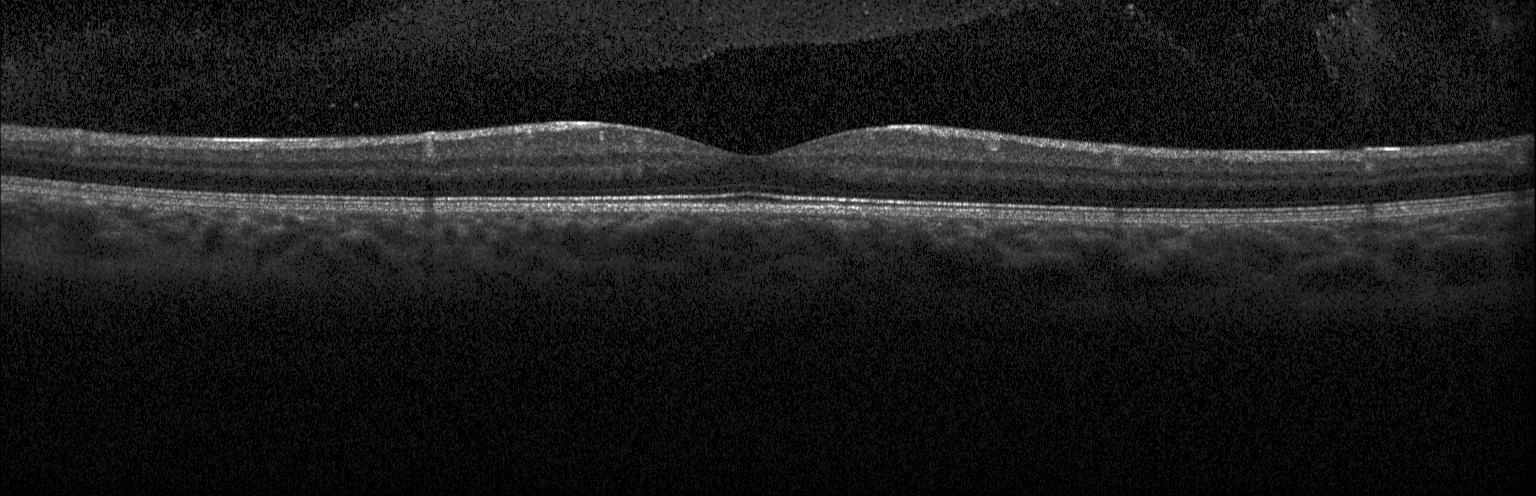

Retinal OCT cross-section
Impression: no choroidal neovascularization, no diabetic macular edema, and no drusen.